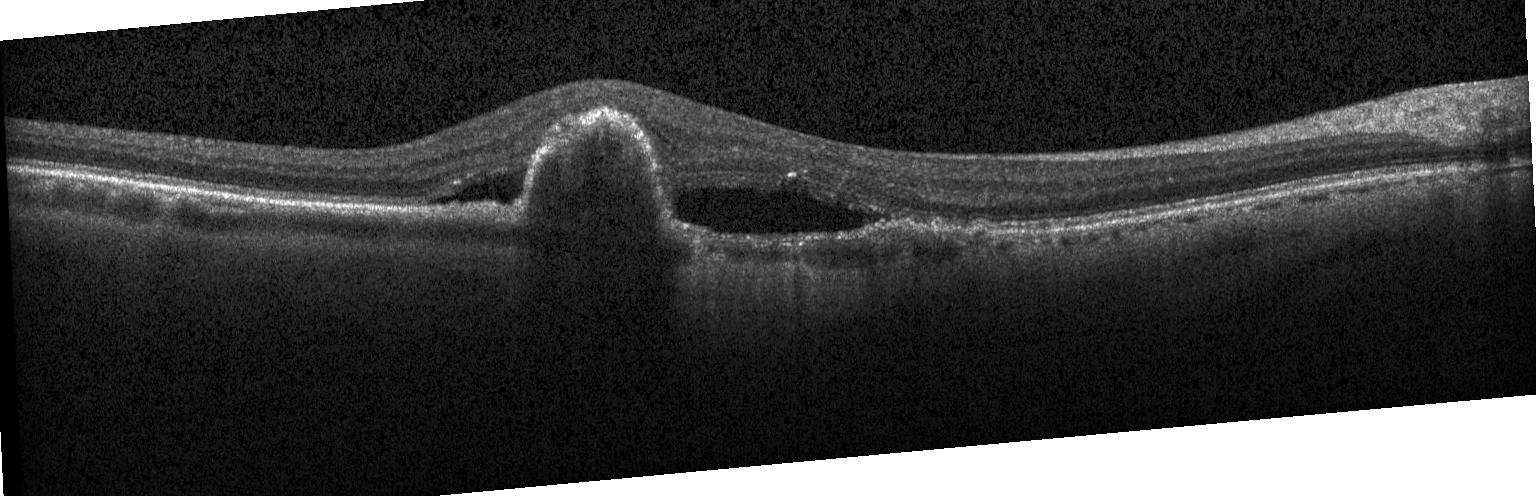
Through the macula. SD-OCT. Optical coherence tomography scan. CNV.